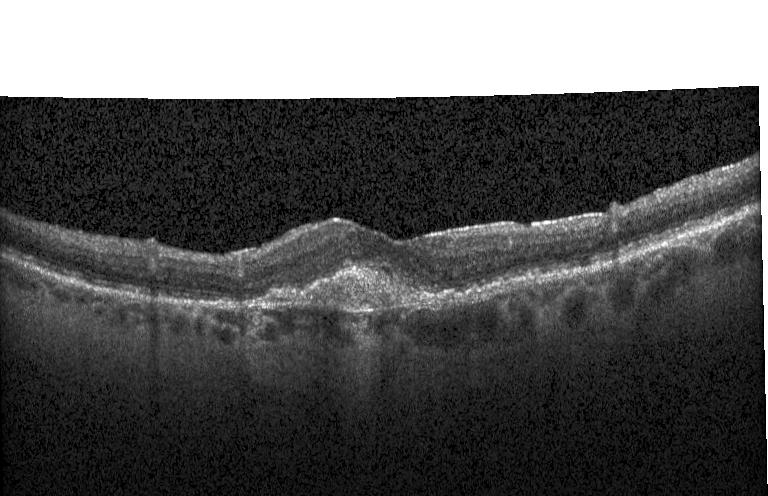

Retinal OCT cross-section showing a choroidal neovascular membrane.